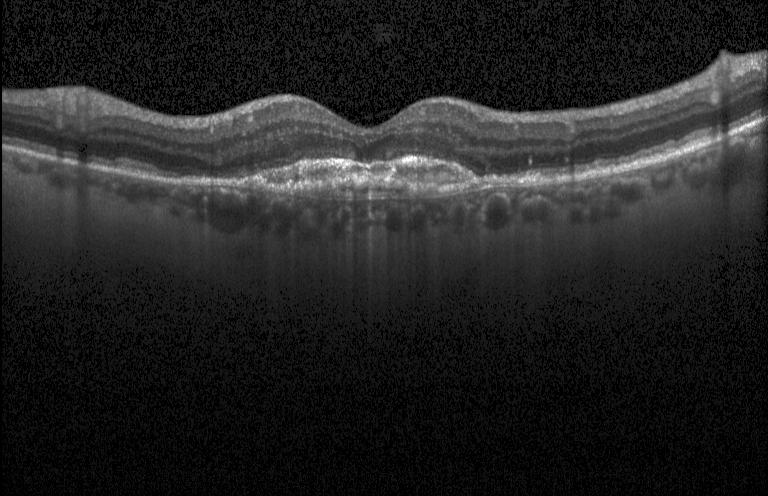

Heidelberg Spectralis OCT system · OCT B-scan · spectral-domain OCT · centered on the fovea — Impression: a choroidal neovascular membrane.